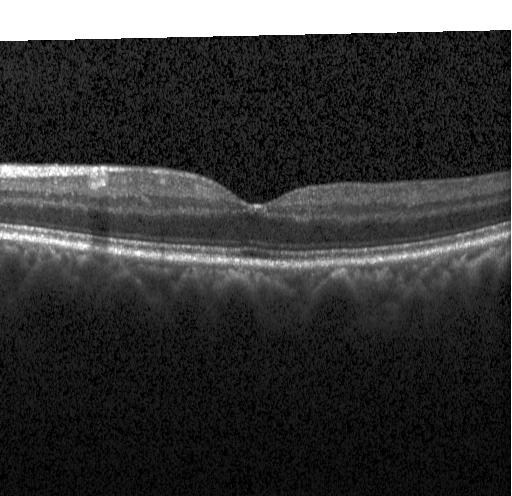
Retinal OCT cross-section · macular scan · acquired on a Heidelberg Spectralis · SD-OCT. Diagnosis: no choroidal neovascularization, no diabetic macular edema, and no drusen.